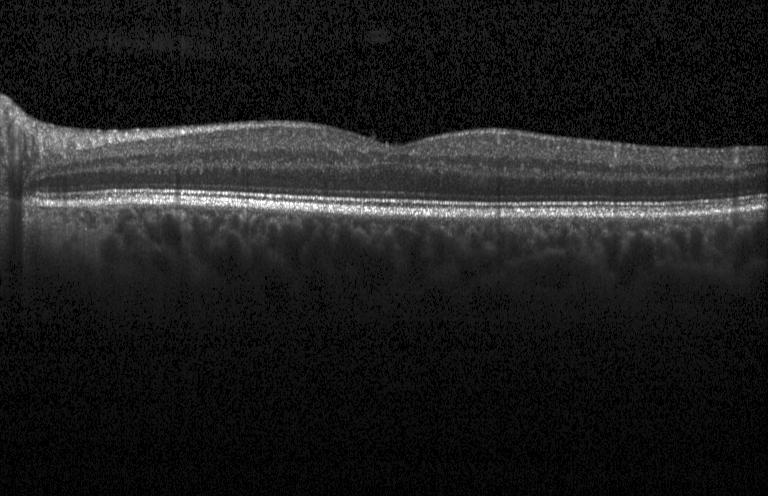

This B-scan demonstrates no evidence of CNV, DME, or drusen.